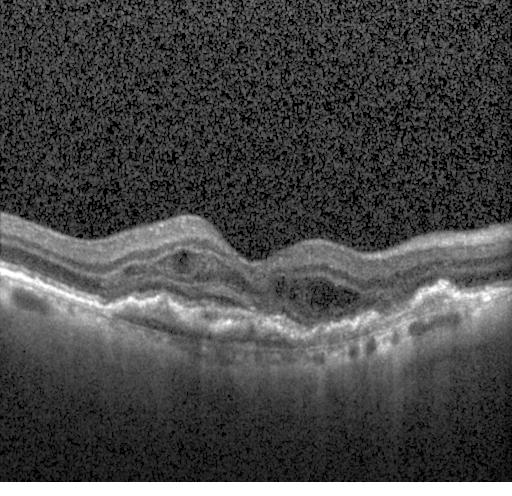

OCT line scan. Impression: CNV.